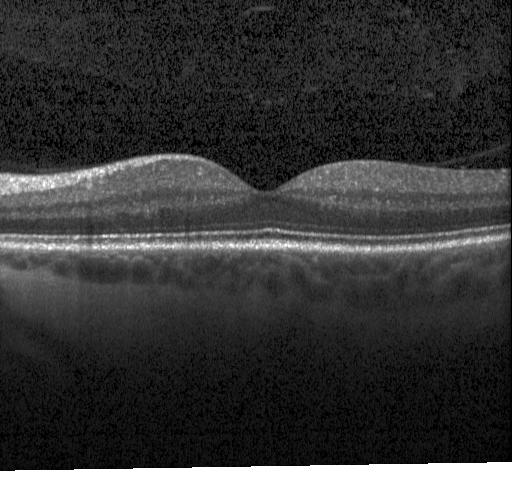

Macular OCT: no CNV, DME, or drusen.